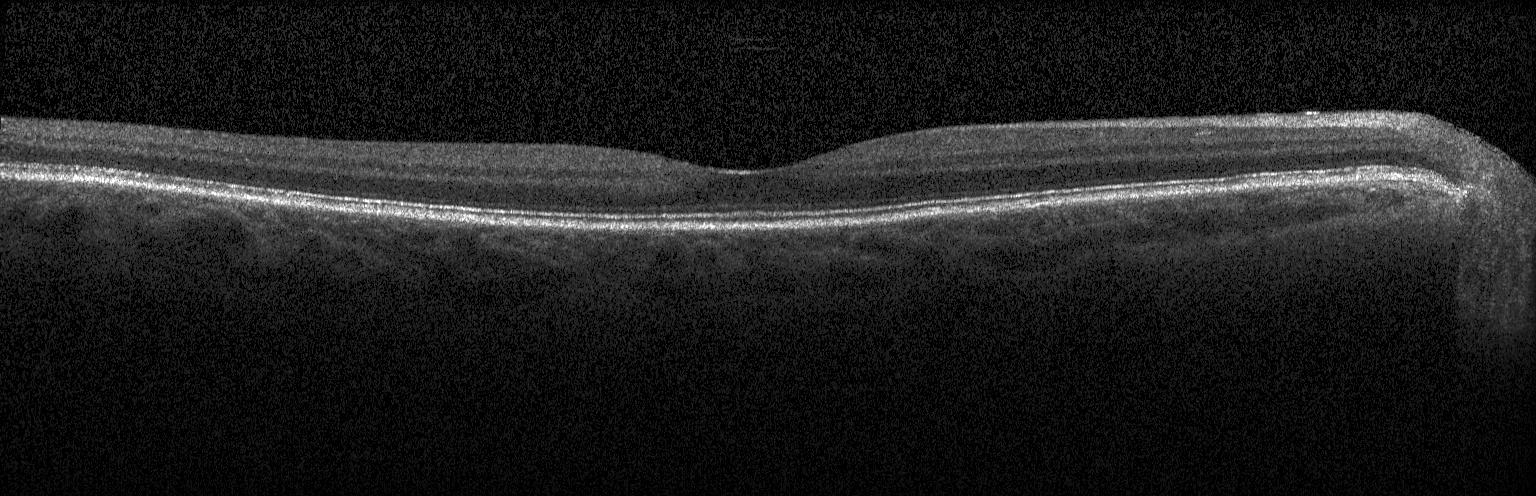

Optical coherence tomography B-scan · centered on the fovea · acquired on a Heidelberg Spectralis · spectral-domain OCT. Dx: neither CNV, DME, nor drusen.